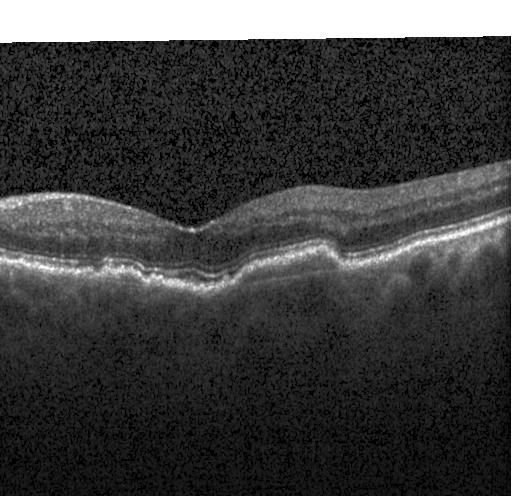 SD-OCT, OCT line scan.
Macular OCT: CNV.